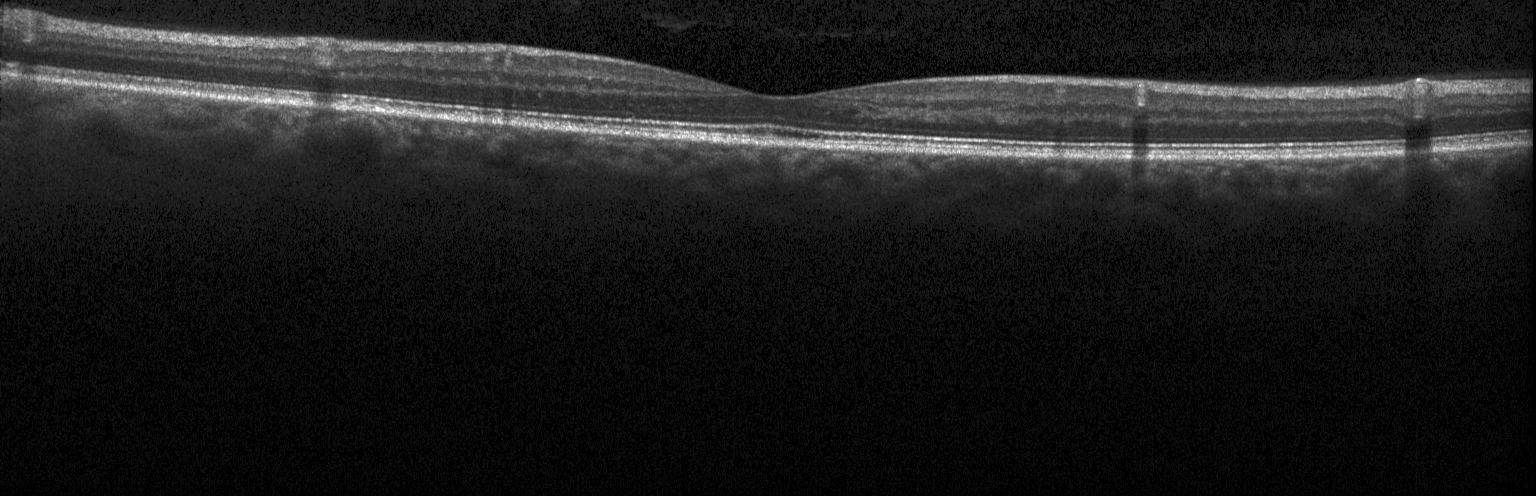
Spectral-domain optical coherence tomography. OCT B-scan. Centered on the fovea — This B-scan demonstrates no evidence of choroidal neovascularization, diabetic macular edema, or drusen.